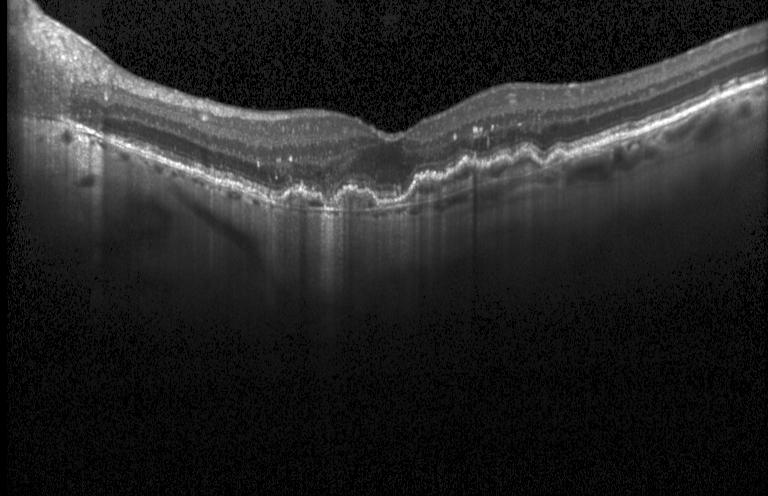
Diagnosis: CNV.